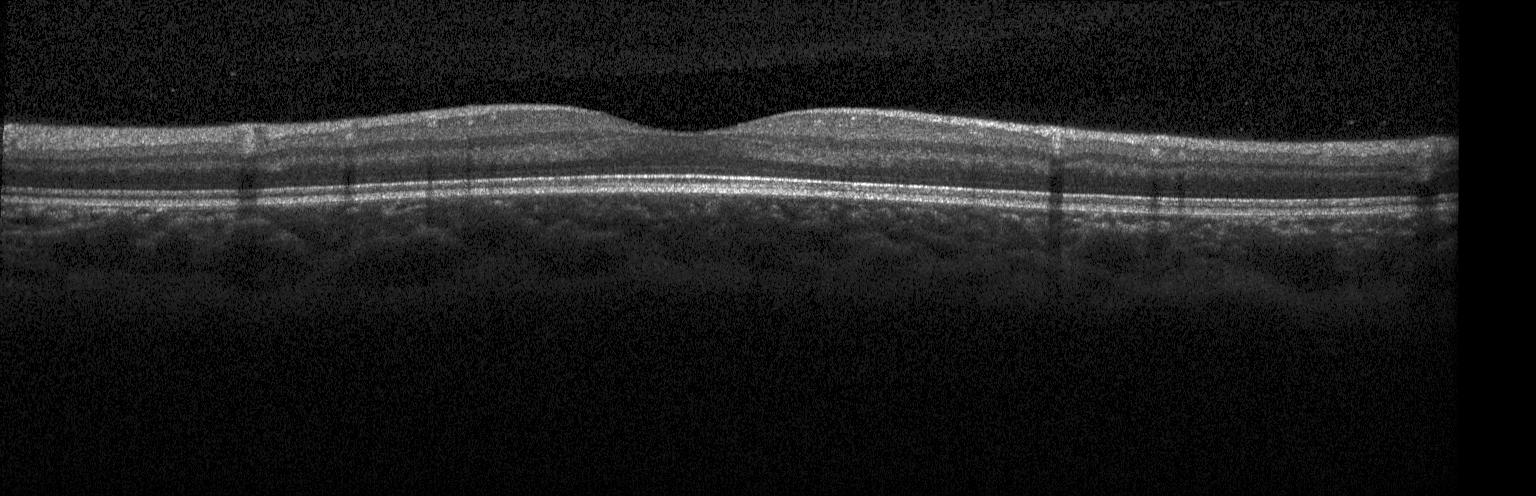

OCT scan showing neither CNV, DME, nor drusen.